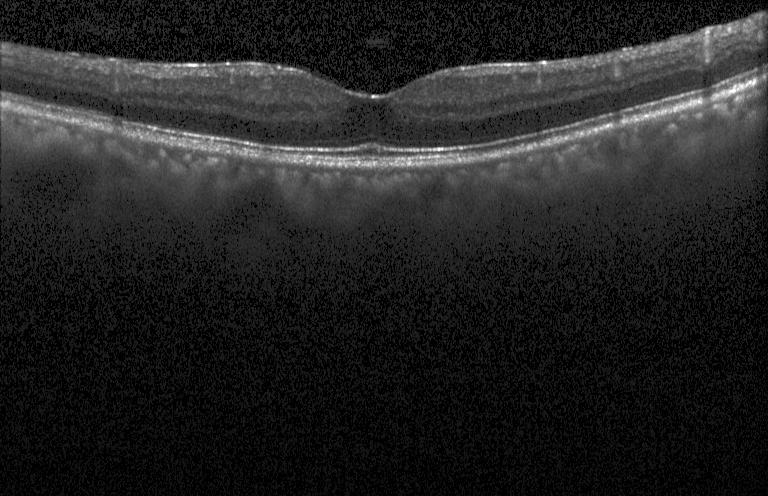 Retinal OCT B-scan · Heidelberg Spectralis.
OCT finding: no choroidal neovascularization, diabetic macular edema, or drusen.